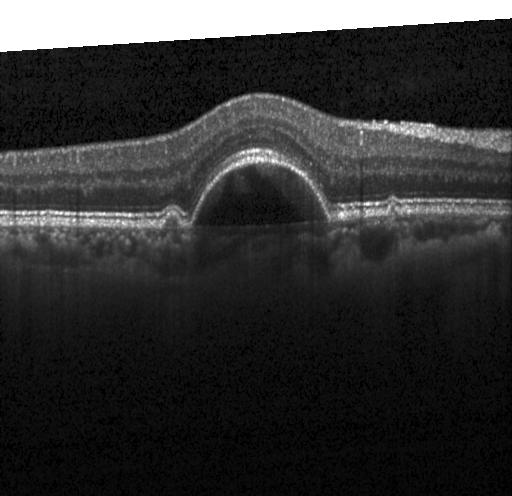

Assessment: a choroidal neovascular membrane.